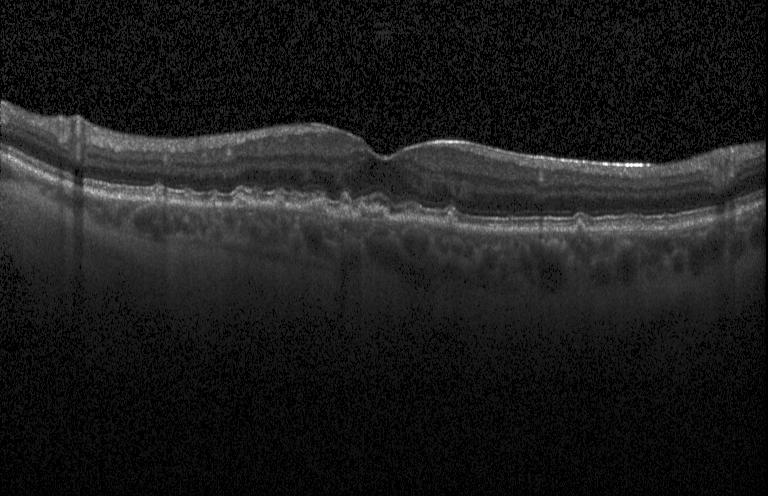

OCT finding: multiple drusen.